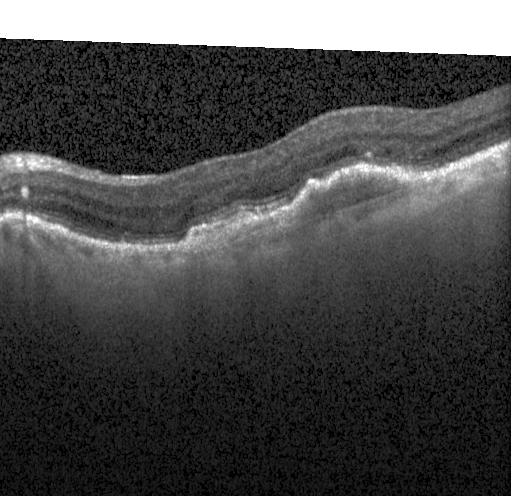

OCT B-scan; spectral-domain OCT.
Finding: a choroidal neovascular membrane.